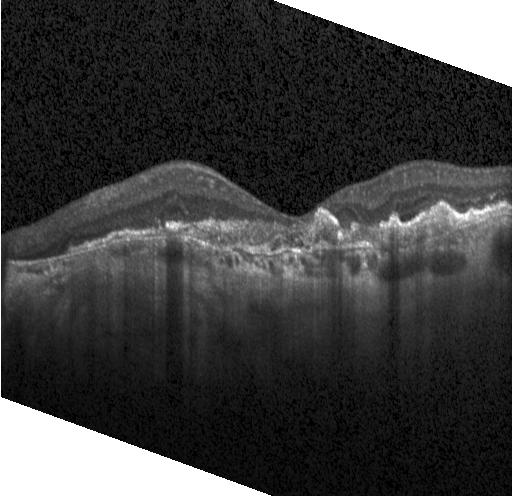
Instrument: Heidelberg Spectralis; optical coherence tomography scan — Diagnosis: a choroidal neovascular membrane.